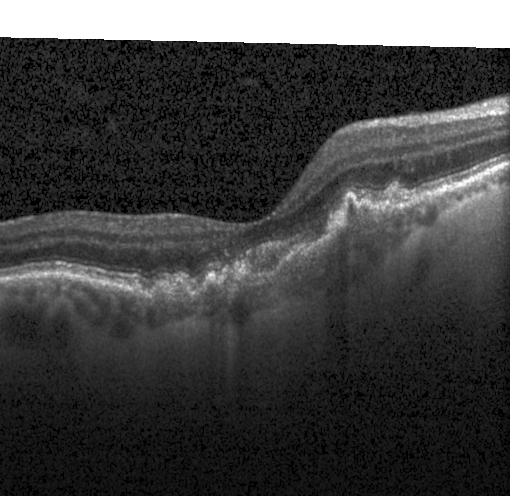

Acquired on a Heidelberg Spectralis · macular scan · OCT B-scan · spectral-domain OCT. Choroidal neovascularization.